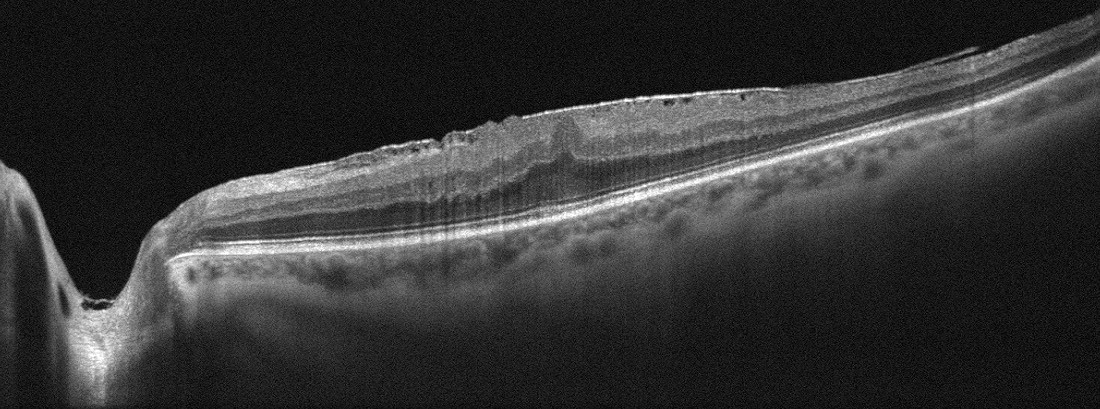

Macular OCT demonstrating ERM.